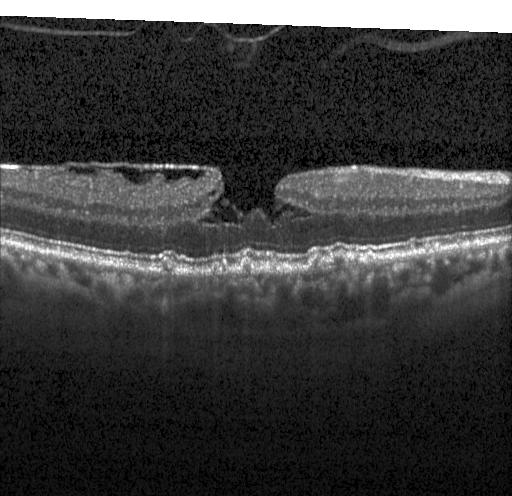

OCT B-scan — Macular OCT: drusen.